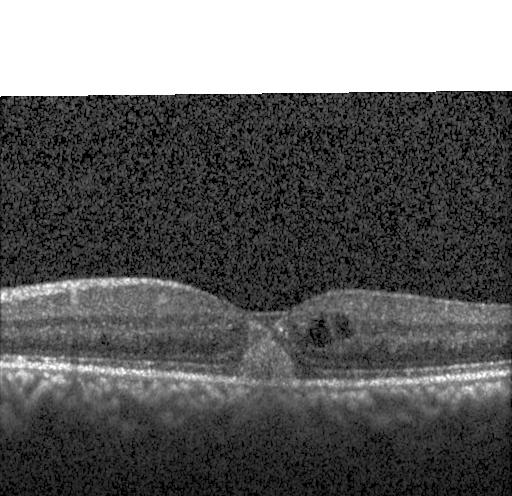

Centered on the fovea. OCT line scan. Spectral-domain OCT. Impression: choroidal neovascularization (CNV).